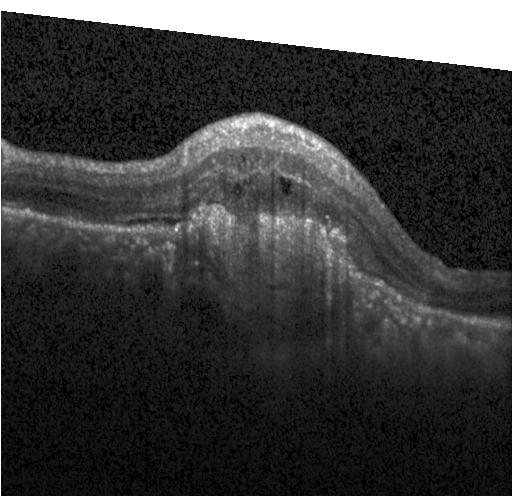

Horizontal scan through the fovea. Optical coherence tomography scan. SD-OCT — Diagnosis: a choroidal neovascular membrane.